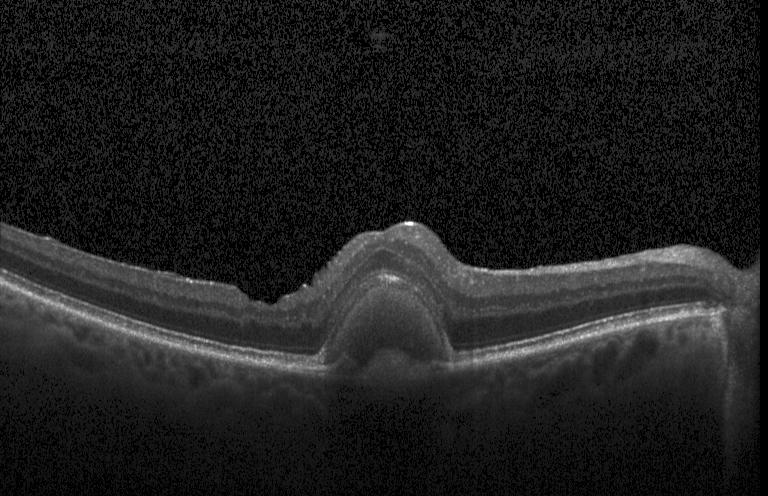

Optical coherence tomography scan.
A choroidal neovascular membrane.